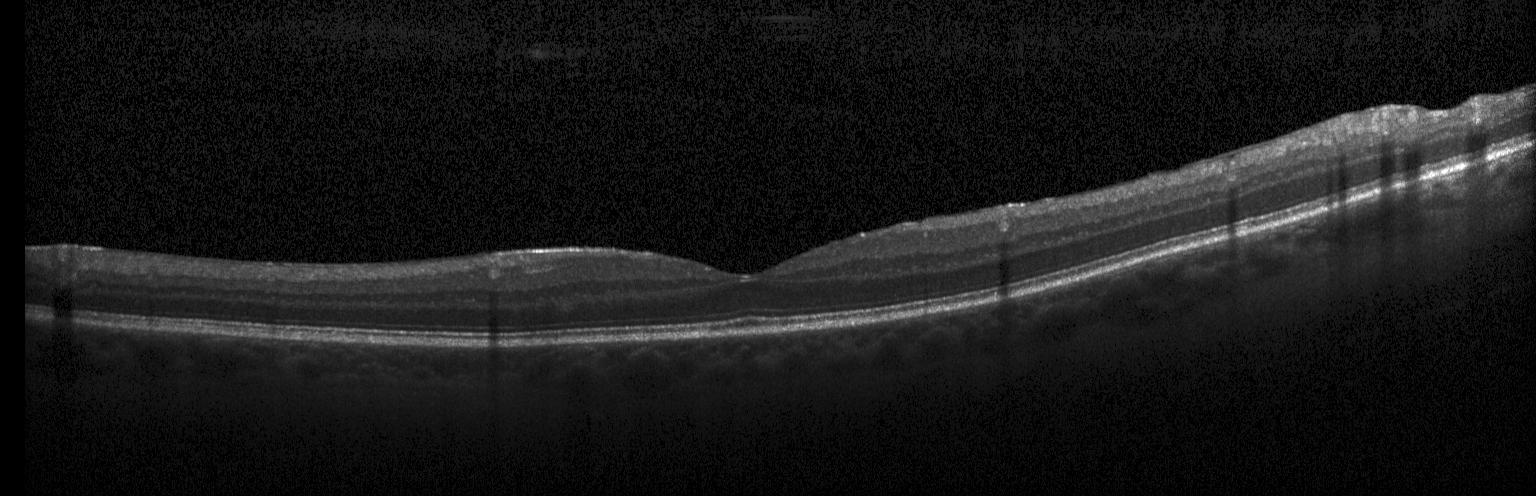

Retinal OCT B-scan — Finding: neither choroidal neovascularization, diabetic macular edema, nor drusen.